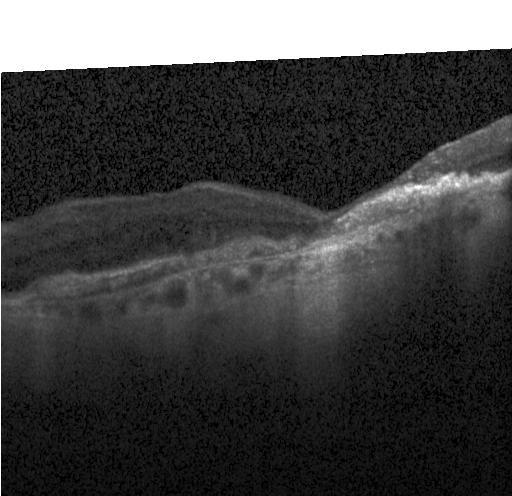 Optical coherence tomography B-scan · macular scan · instrument: Heidelberg Spectralis · SD-OCT.
Impression: a choroidal neovascular membrane.